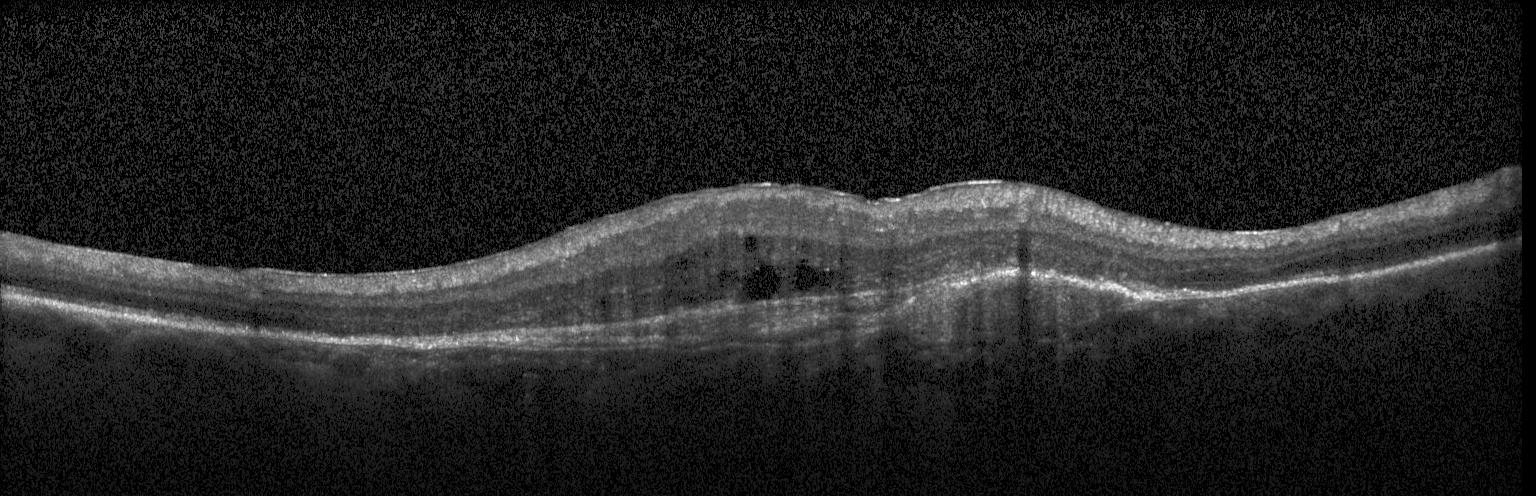
This B-scan demonstrates choroidal neovascularization (CNV).